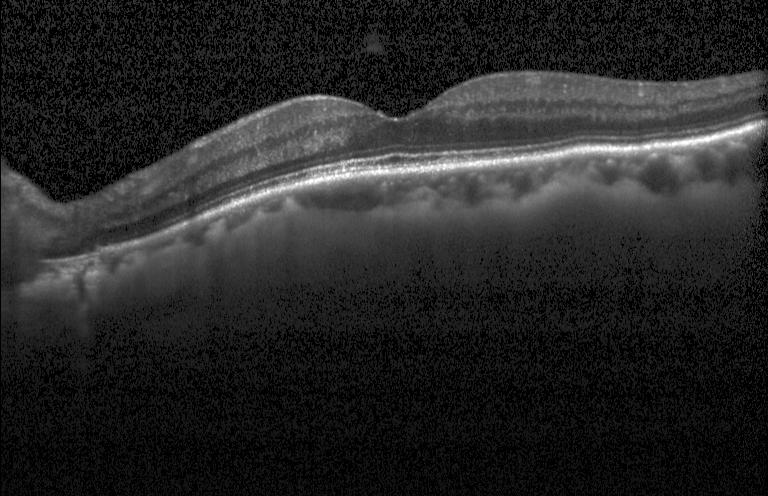
Dx: no evidence of choroidal neovascularization, diabetic macular edema, or drusen.